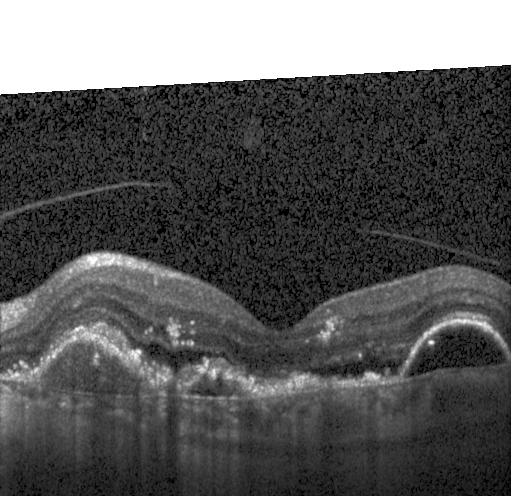
Through the macula, SD-OCT, retinal OCT cross-section, Heidelberg Spectralis.
Finding: a choroidal neovascular membrane.